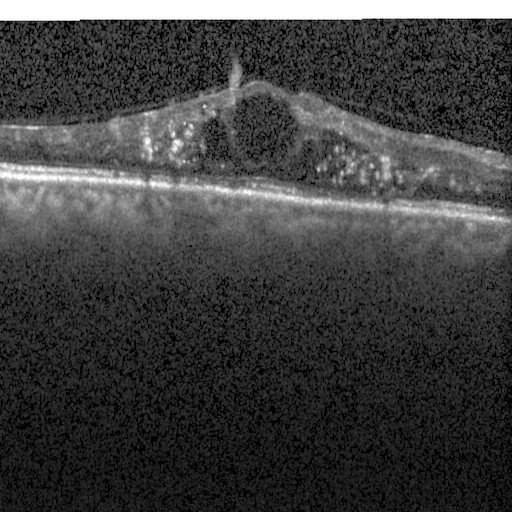 OCT scan showing diabetic macular edema.